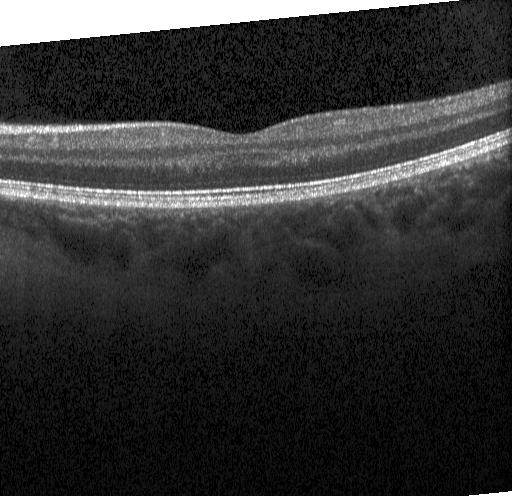
Dx: no evidence of choroidal neovascularization, diabetic macular edema, or drusen.